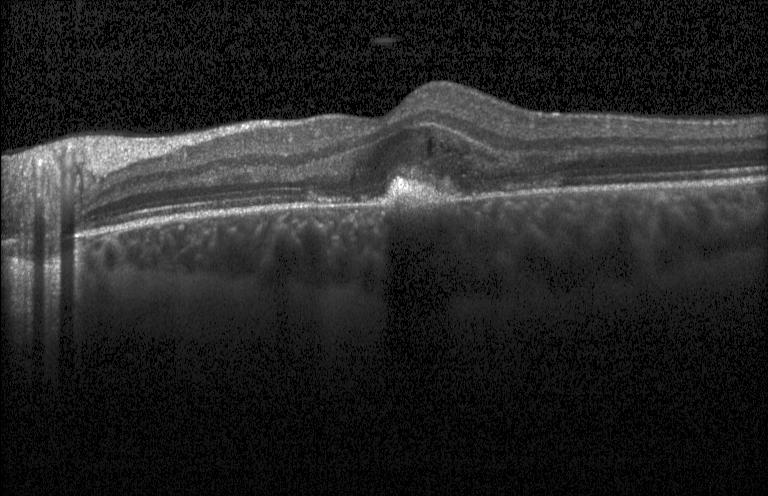
Optical coherence tomography scan. Heidelberg Spectralis. Spectral-domain optical coherence tomography — Macular OCT: a choroidal neovascular membrane.